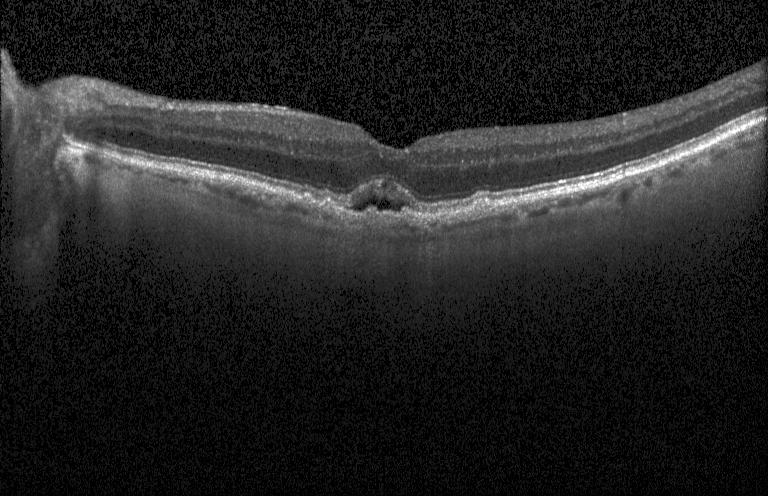
Retinal OCT B-scan
Impression: CNV.